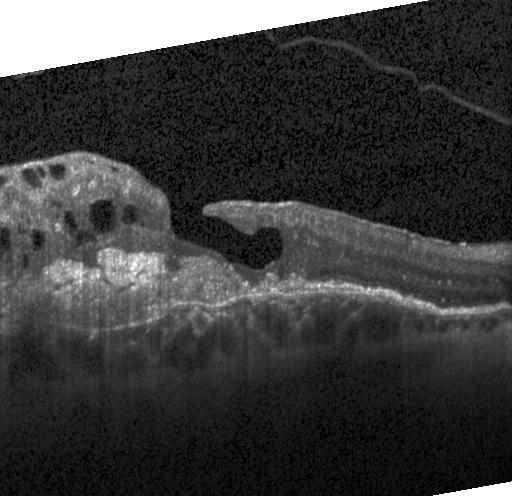
OCT line scan. Finding: CNV.